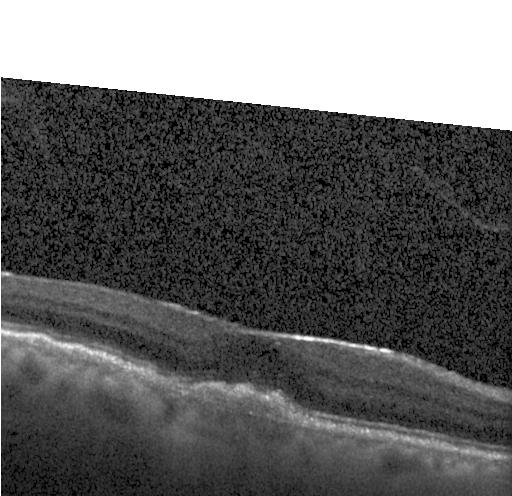
SD-OCT, OCT line scan, Heidelberg Spectralis OCT system. The scan shows CNV.